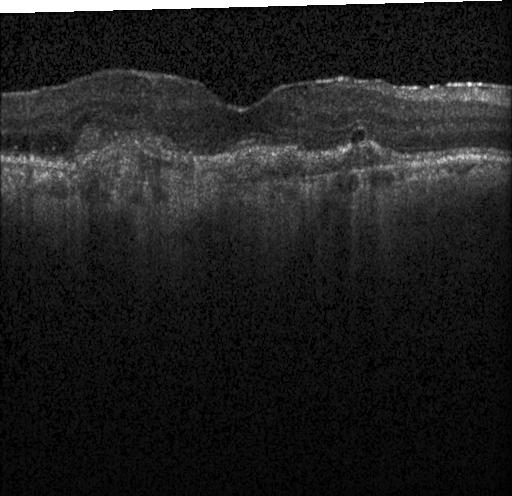 Acquired on a Heidelberg Spectralis · optical coherence tomography scan.
Diagnosis: a choroidal neovascular membrane.